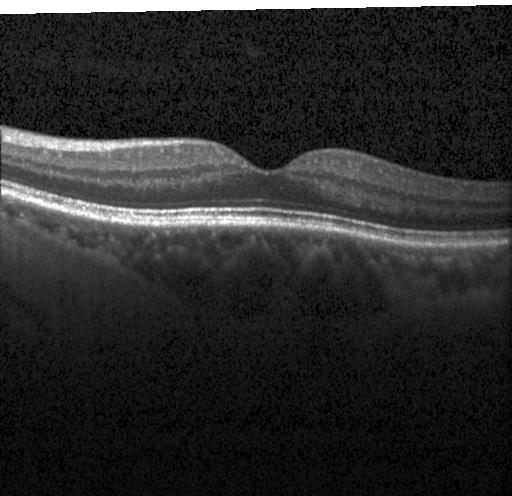 Macular OCT demonstrating neither choroidal neovascularization, diabetic macular edema, nor drusen.